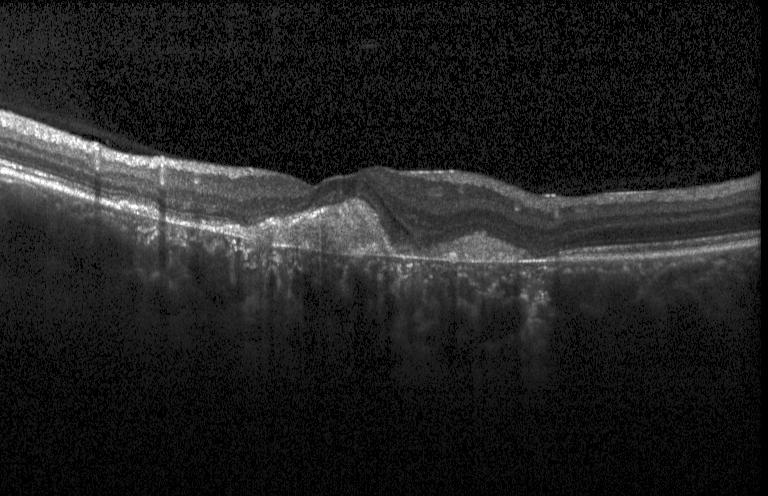 Horizontal scan through the fovea; spectral-domain optical coherence tomography; retinal OCT cross-section. Dx: CNV.